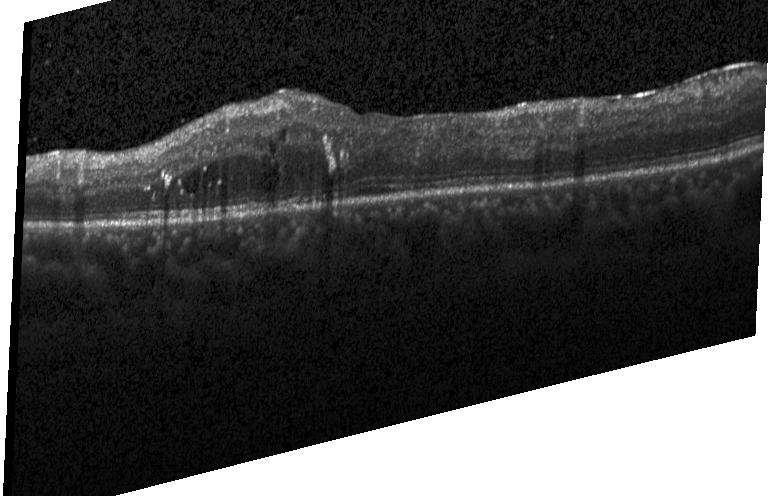
OCT line scan.
Diagnosis: DME.